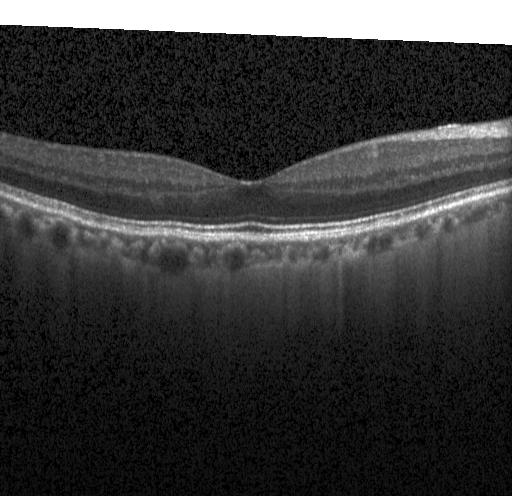
Optical coherence tomography scan, spectral-domain optical coherence tomography. Finding: neither choroidal neovascularization, diabetic macular edema, nor drusen.